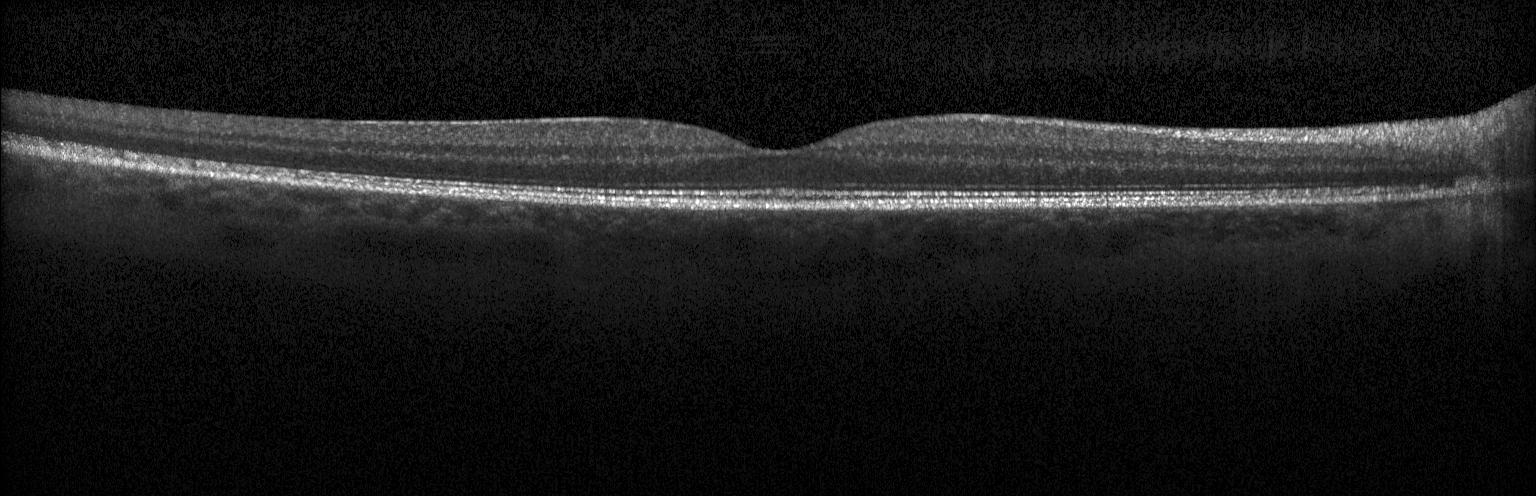
The scan shows no CNV, no DME, and no drusen.